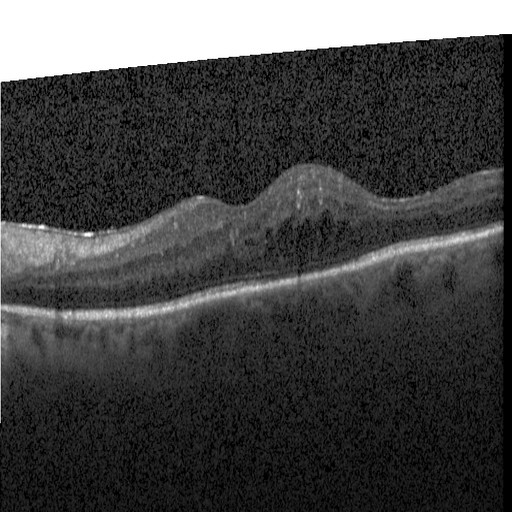
Macular OCT: DME.